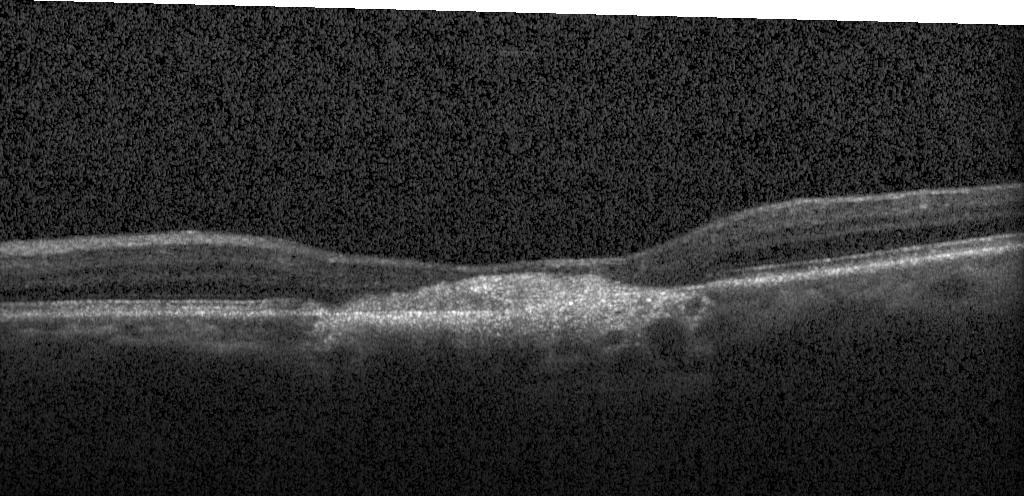
A choroidal neovascular membrane.